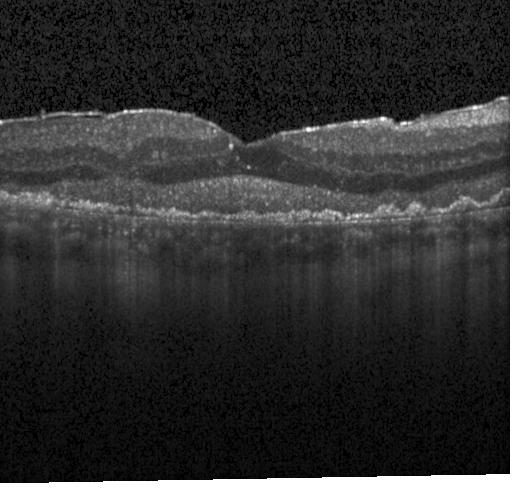
Macular OCT: a choroidal neovascular membrane.